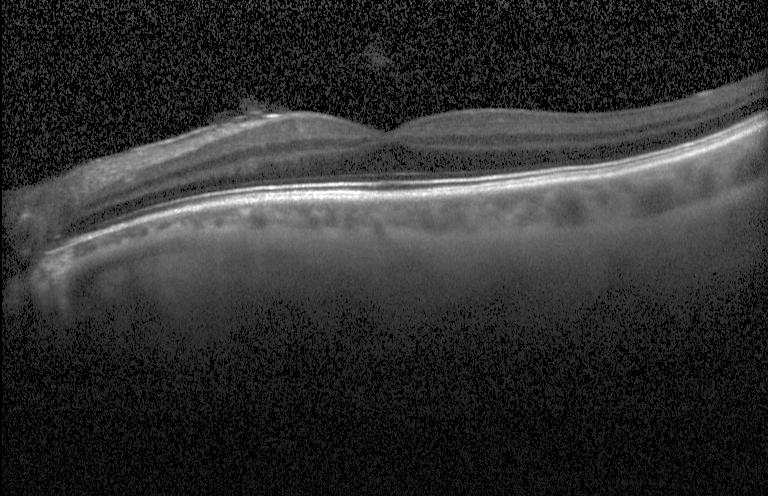
SD-OCT. OCT line scan. The scan shows neither CNV, DME, nor drusen.